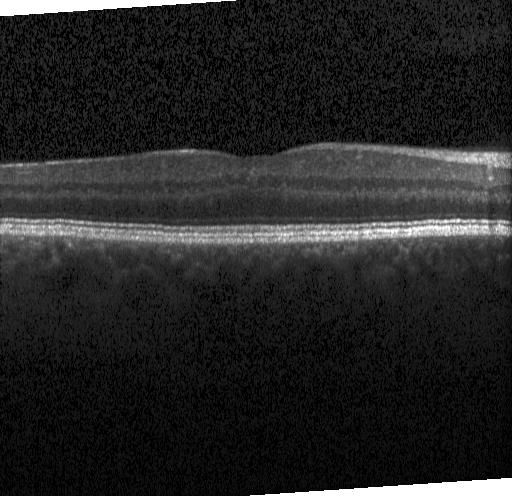 Acquired on a Heidelberg Spectralis. Spectral-domain OCT. Optical coherence tomography B-scan. Through the macula
Macular OCT: neither choroidal neovascularization, diabetic macular edema, nor drusen.